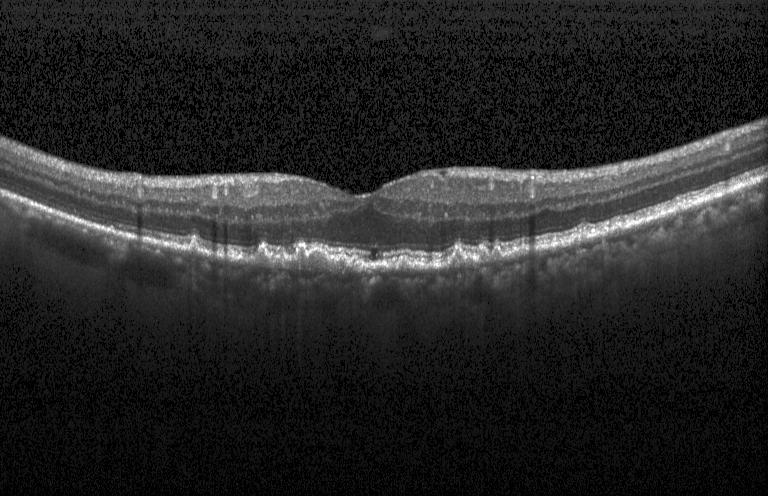

Retinal OCT B-scan · centered on the fovea · Heidelberg Spectralis OCT system — Dx: drusen.